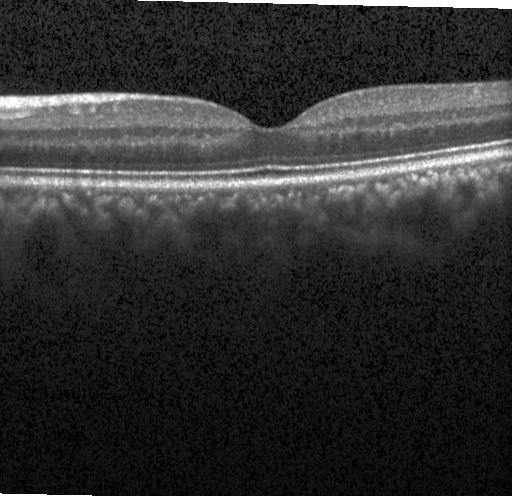
OCT line scan. Horizontal scan through the fovea. Heidelberg Spectralis. Spectral-domain optical coherence tomography. Impression: no choroidal neovascularization, diabetic macular edema, or drusen.